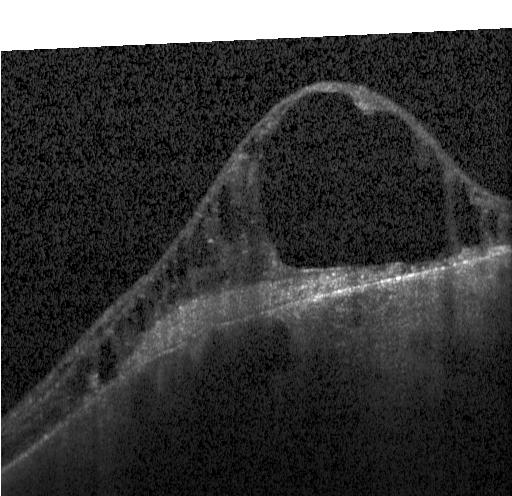
Horizontal scan through the fovea, optical coherence tomography scan, spectral-domain optical coherence tomography.
Impression: a choroidal neovascular membrane.